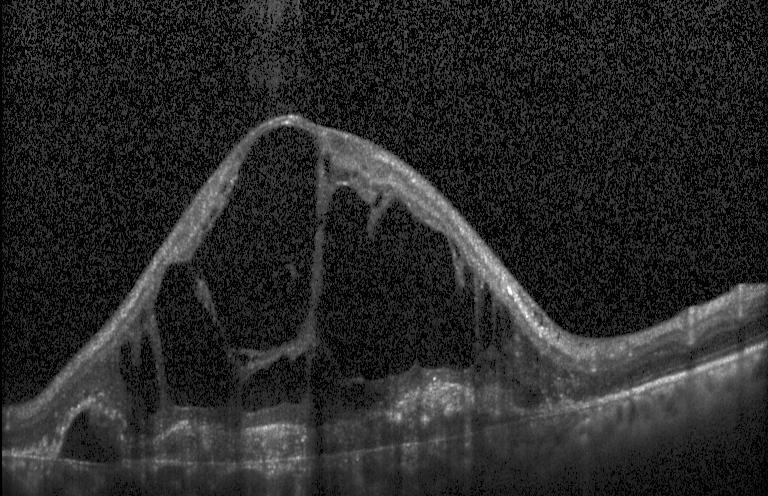
Retinal OCT B-scan; spectral-domain optical coherence tomography; horizontal scan through the fovea; acquired on a Heidelberg Spectralis
Finding: a choroidal neovascular membrane.